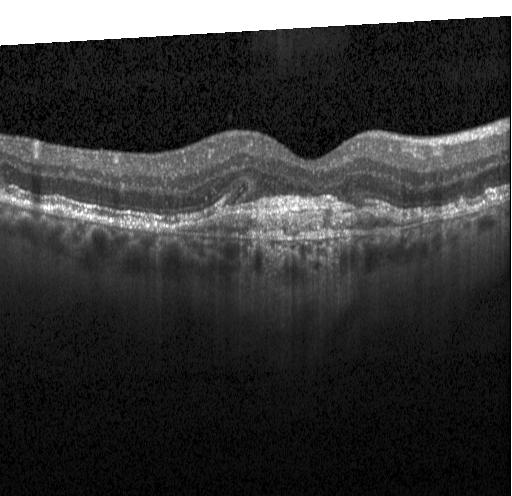 Diagnosis: a choroidal neovascular membrane.